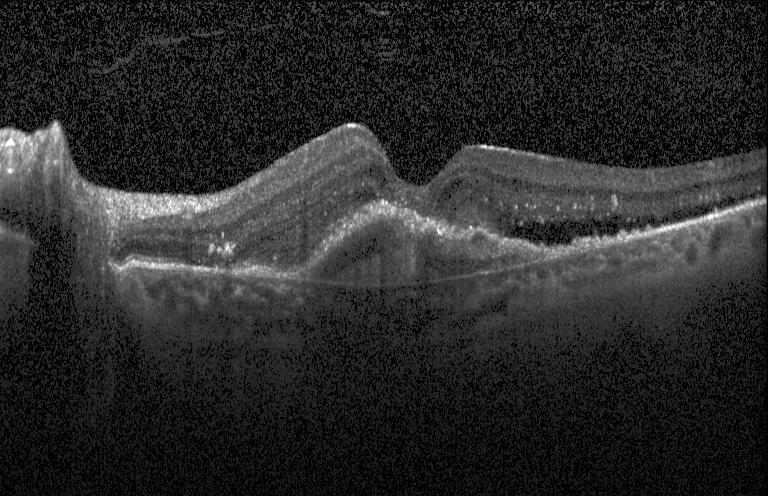
Spectral-domain OCT B-scan: a choroidal neovascular membrane.